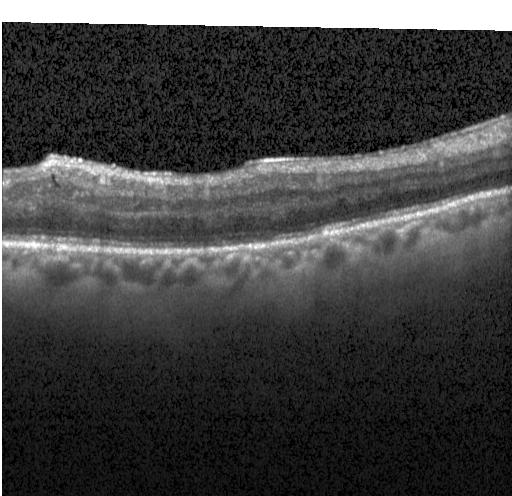 Retinal OCT B-scan — Finding: diabetic macular edema (DME).